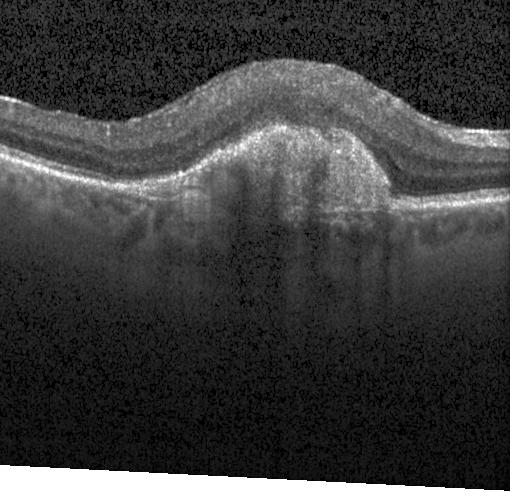 Optical coherence tomography B-scan · horizontal scan through the fovea.
Finding: choroidal neovascularization (CNV).